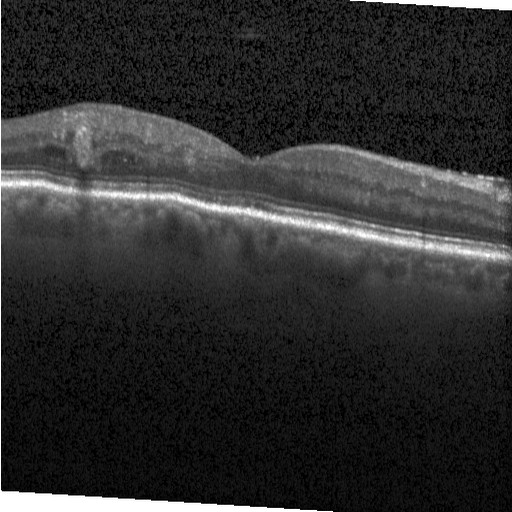
Spectral-domain OCT · retinal OCT cross-section · centered on the fovea — Diagnosis: diabetic macular edema (DME).